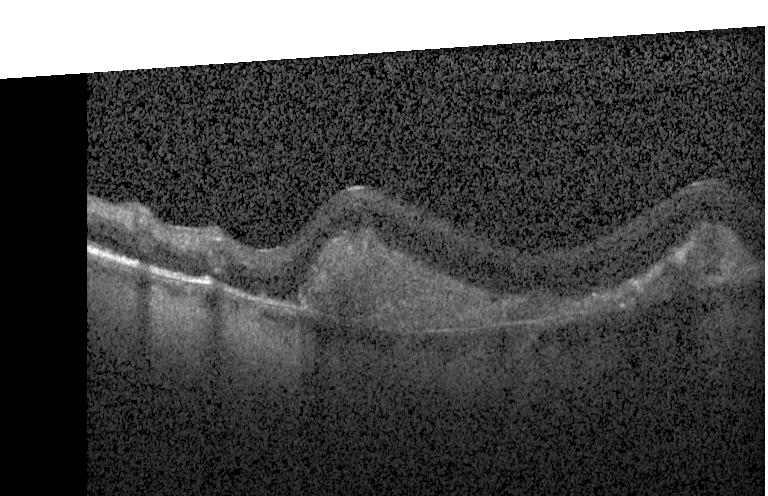

Centered on the fovea. Instrument: Heidelberg Spectralis. Spectral-domain optical coherence tomography. Retinal OCT cross-section. Diagnosis: a choroidal neovascular membrane.